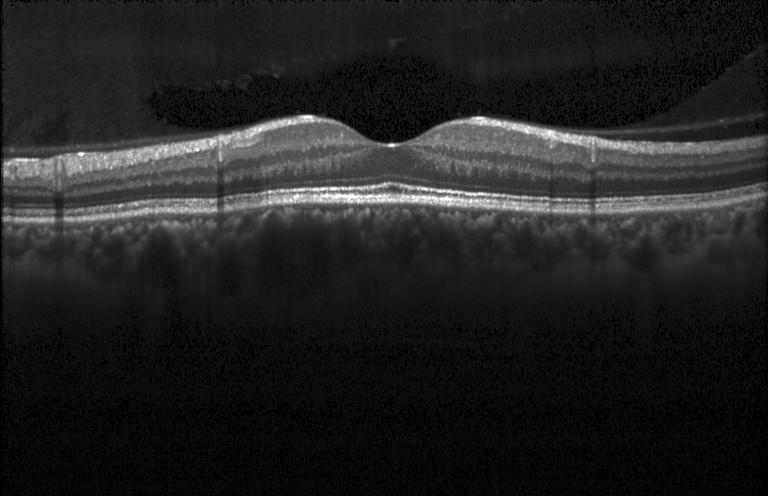

Impression: no evidence of CNV, DME, or drusen.